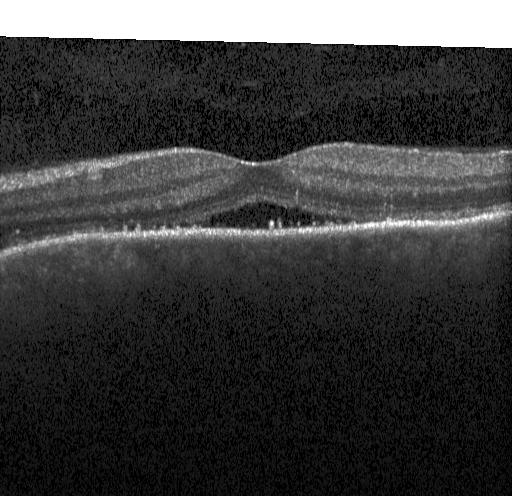

OCT line scan. Heidelberg Spectralis — Dx: a choroidal neovascular membrane.